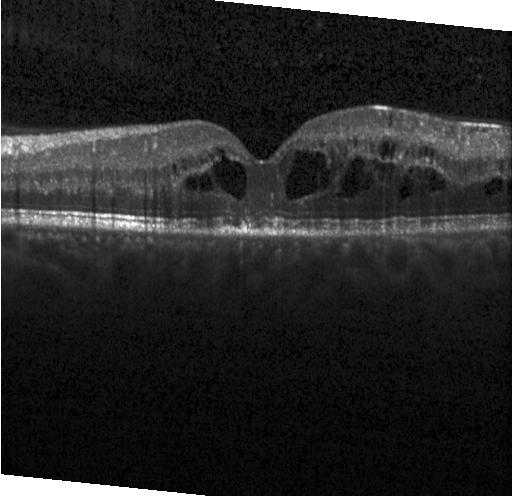 Impression: diabetic macular edema (DME).